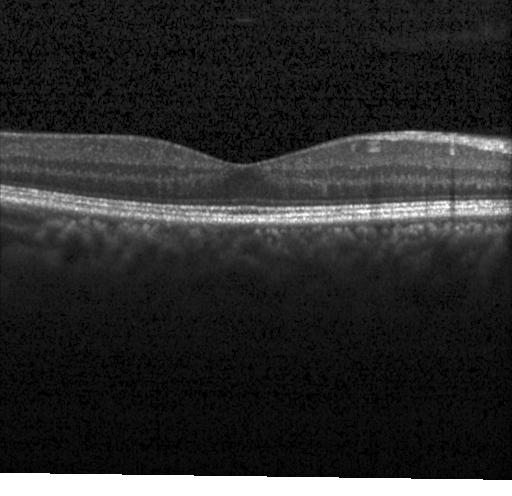
Macular scan. OCT line scan — Diagnosis: no CNV, no DME, and no drusen.